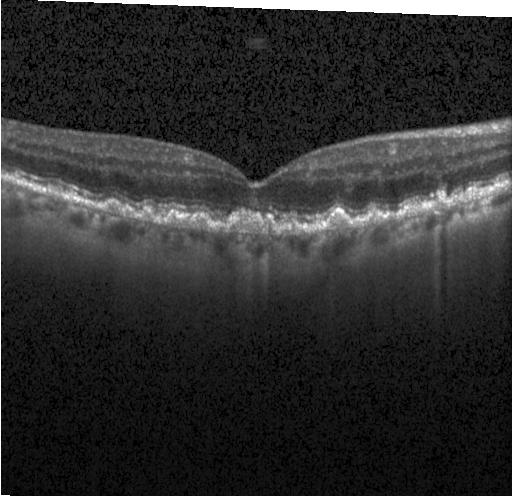

Finding: drusen.